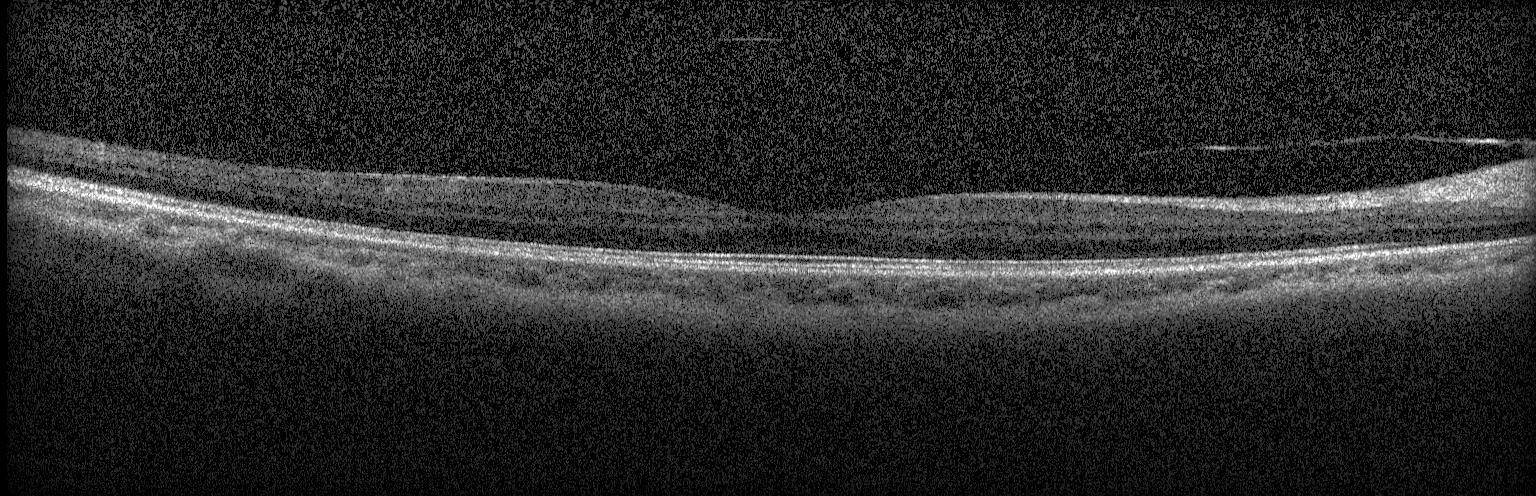
Acquired on a Heidelberg Spectralis · retinal OCT B-scan · spectral-domain optical coherence tomography · through the macula
Diagnosis: no evidence of choroidal neovascularization, diabetic macular edema, or drusen.